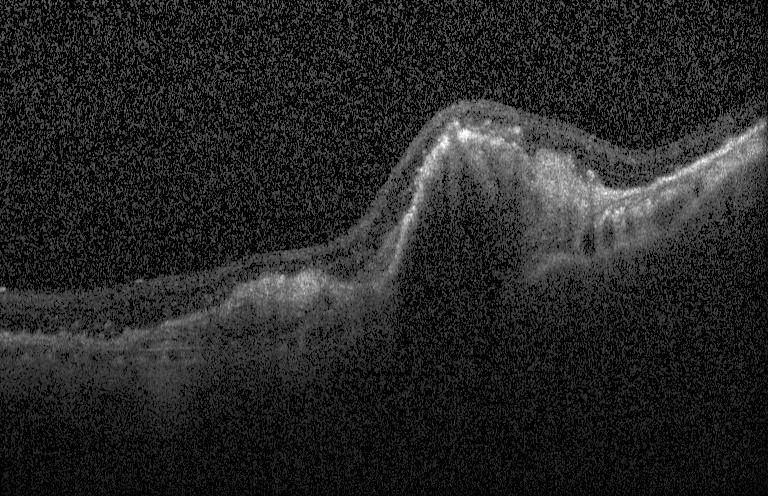 Diagnosis: CNV.